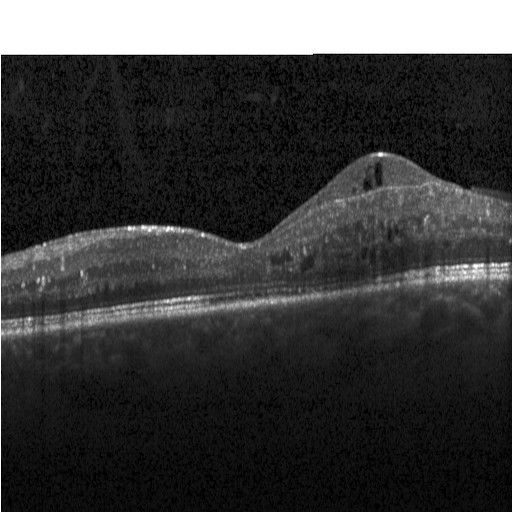

Heidelberg Spectralis OCT system · optical coherence tomography scan · SD-OCT. The scan shows diabetic macular edema (DME).